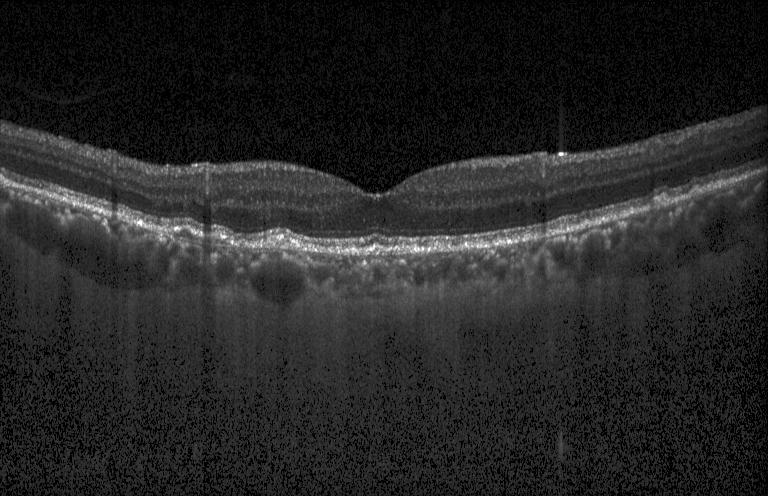

Retinal OCT cross-section · macular scan · instrument: Heidelberg Spectralis.
Impression: multiple drusen.